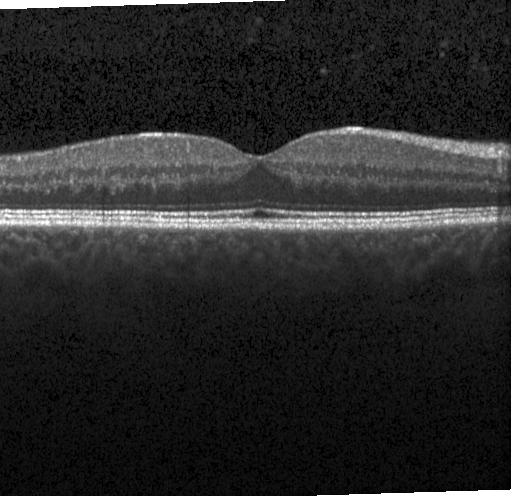
OCT B-scan.
This B-scan demonstrates no CNV, DME, or drusen.